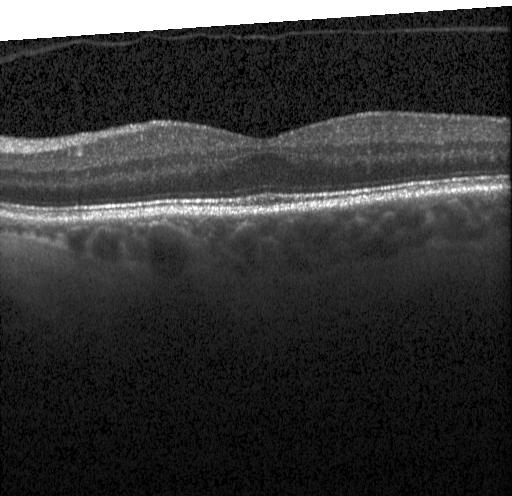

Spectral-domain OCT · Heidelberg Spectralis · retinal OCT cross-section.
Diagnosis: no evidence of choroidal neovascularization, diabetic macular edema, or drusen.